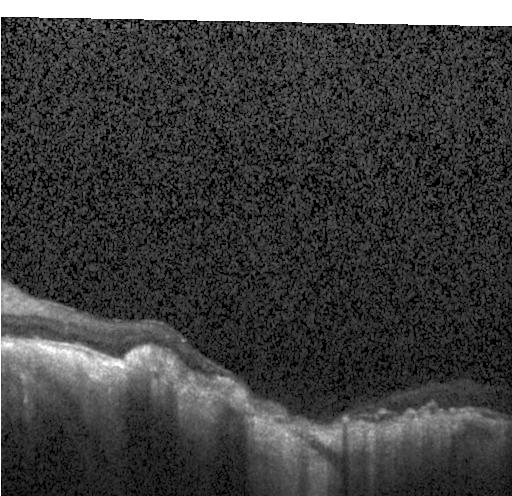 Diagnosis: choroidal neovascularization (CNV).